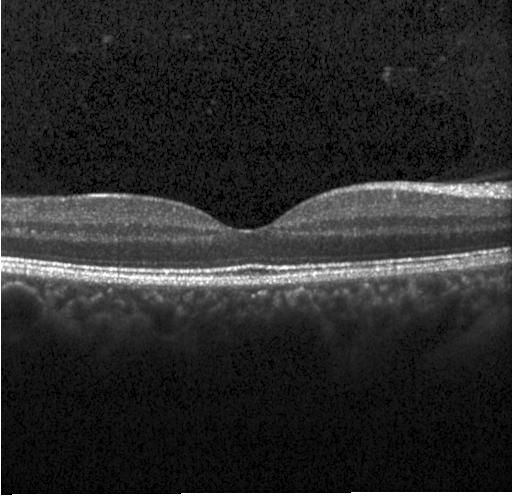
Instrument: Heidelberg Spectralis · optical coherence tomography scan · horizontal scan through the fovea · SD-OCT — Assessment: neither choroidal neovascularization, diabetic macular edema, nor drusen.